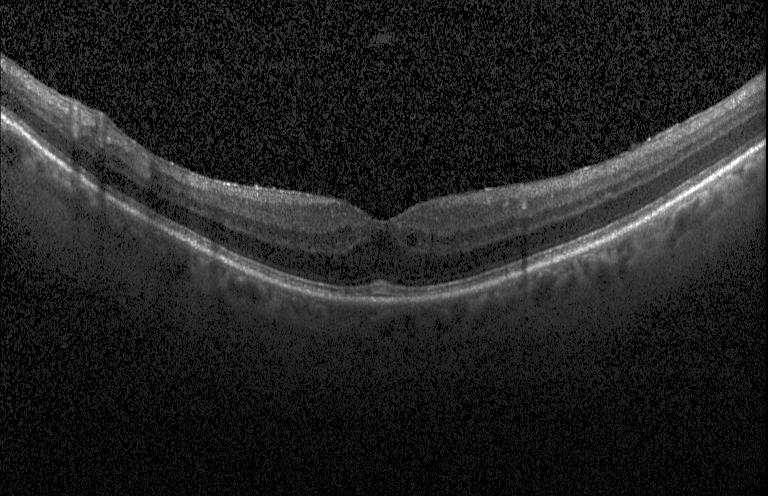
OCT finding: diabetic macular edema.